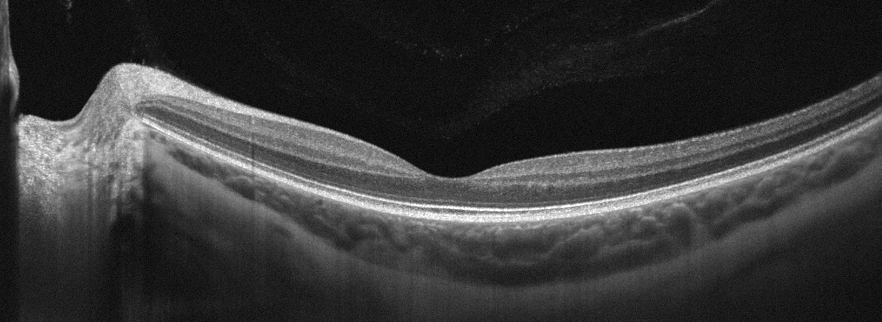

Macular scan; Optovue Avanti RTVue XR; left eye; retinal OCT B-scan
Dx: absence of AMD, DME, ERM, RAO, RVO, and vitreomacular interface disease.